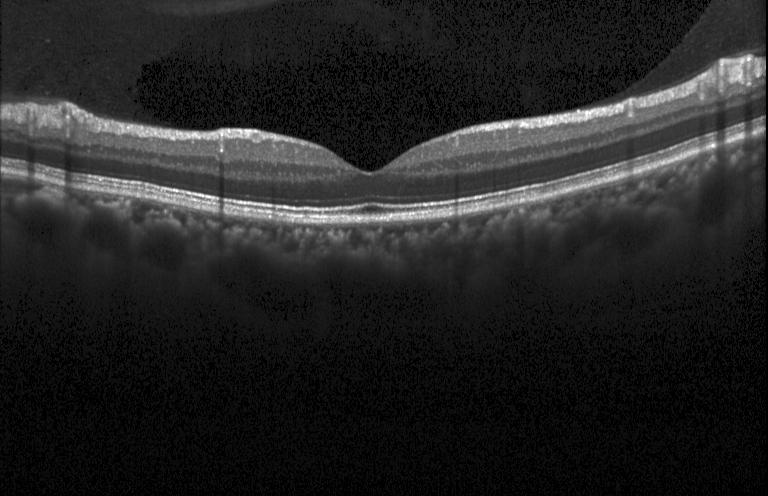
Optical coherence tomography scan · instrument: Heidelberg Spectralis
This B-scan demonstrates no CNV, no DME, and no drusen.